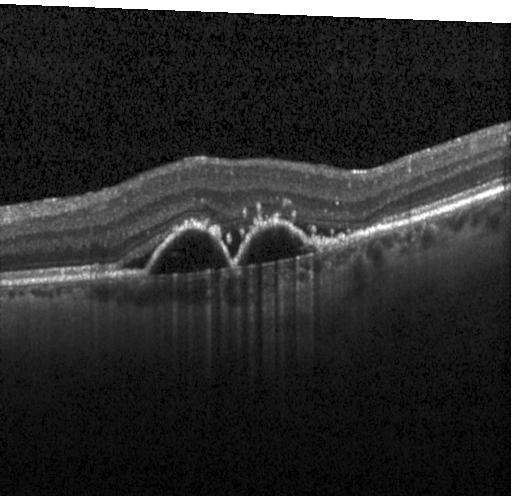
Spectral-domain optical coherence tomography; OCT line scan; Heidelberg Spectralis
Diagnosis: a choroidal neovascular membrane.